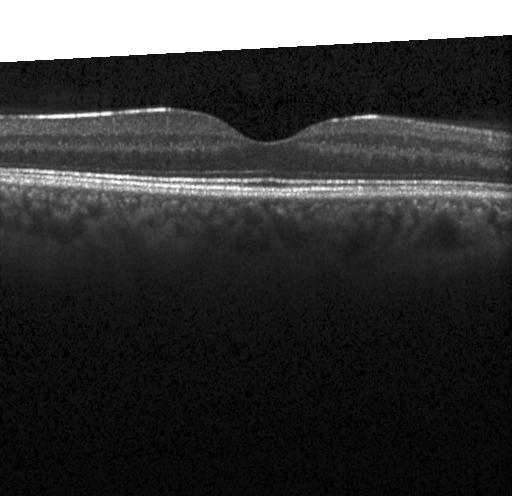
Acquired on a Heidelberg Spectralis · spectral-domain optical coherence tomography · OCT B-scan — Macular OCT: neither CNV, DME, nor drusen.